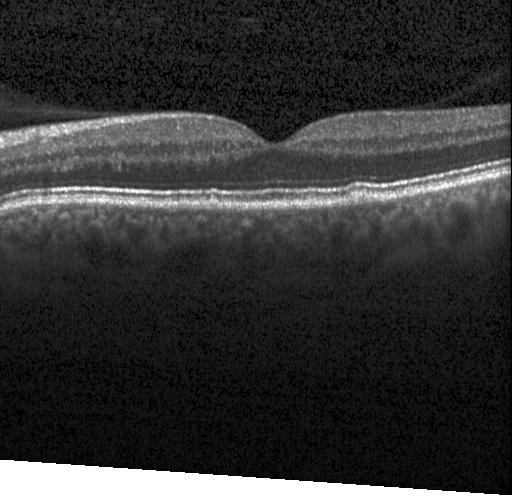
OCT B-scan; instrument: Heidelberg Spectralis; horizontal scan through the fovea; spectral-domain optical coherence tomography.
Dx: multiple drusen.